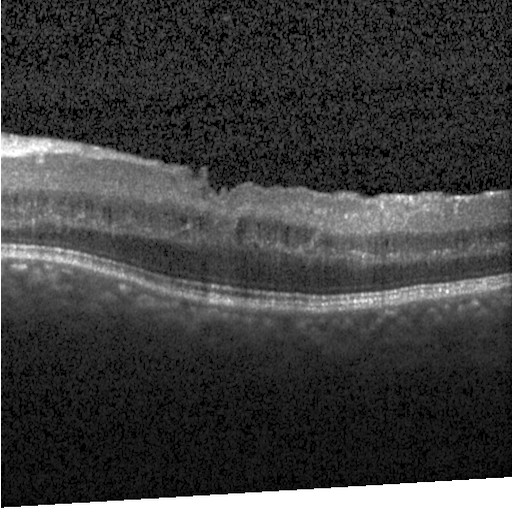
Heidelberg Spectralis · retinal OCT B-scan · SD-OCT · centered on the fovea.
Diagnosis: diabetic macular edema (DME).